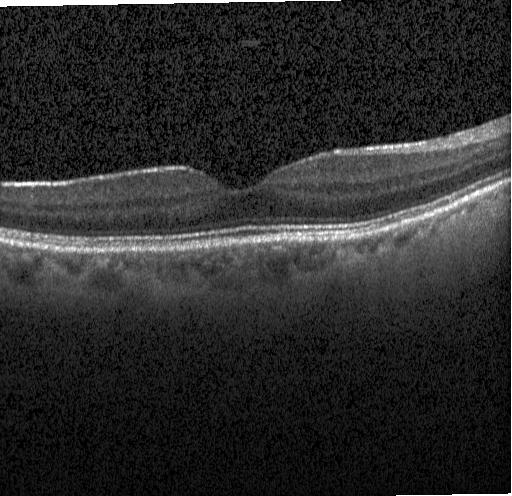 Retinal OCT cross-section, centered on the fovea, spectral-domain OCT, Heidelberg Spectralis — Macular OCT: no CNV, DME, or drusen.